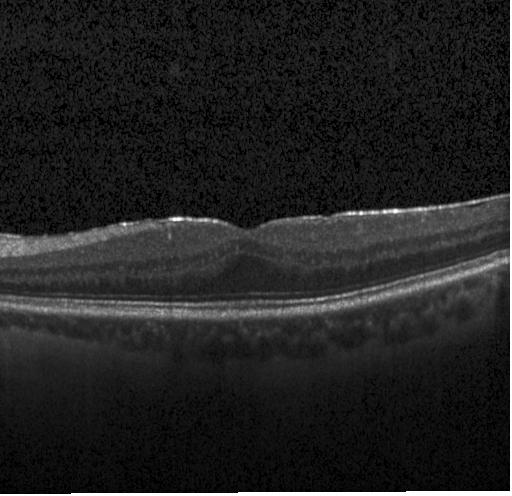 Dx: neither choroidal neovascularization, diabetic macular edema, nor drusen.